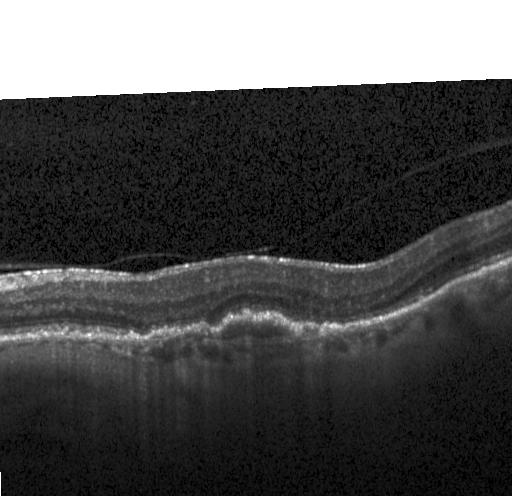 Fovea-centered · OCT B-scan · instrument: Heidelberg Spectralis
Macular OCT: choroidal neovascularization.